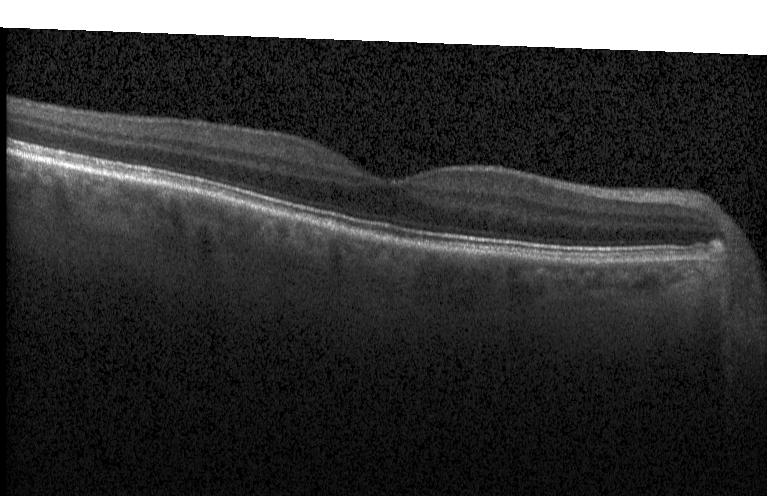
OCT line scan
This B-scan demonstrates no choroidal neovascularization, no diabetic macular edema, and no drusen.